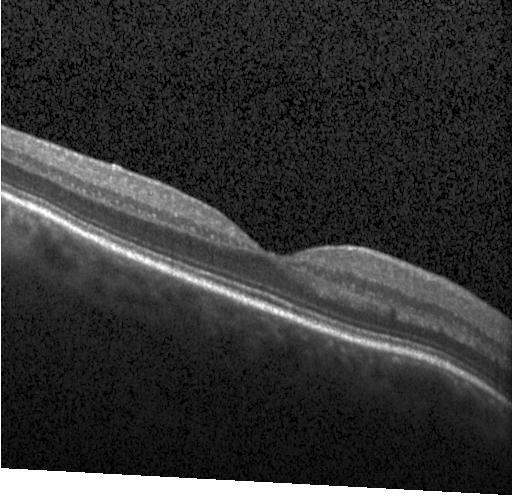
Spectral-domain OCT B-scan: no choroidal neovascularization, no diabetic macular edema, and no drusen.